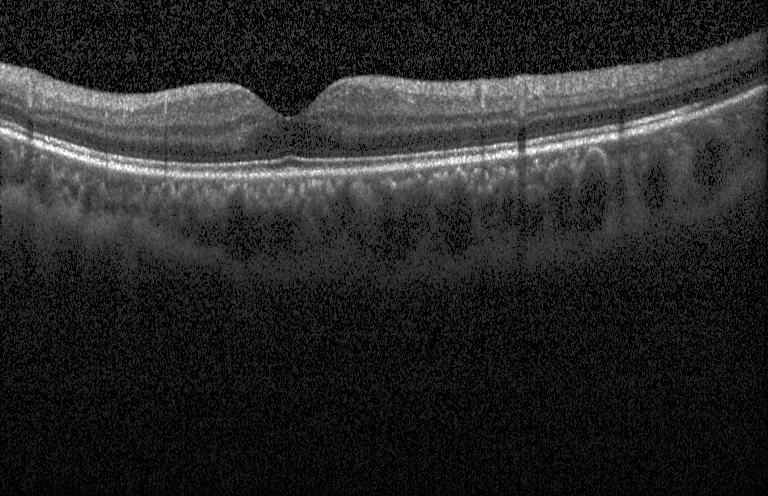 Impression: no evidence of choroidal neovascularization, diabetic macular edema, or drusen.